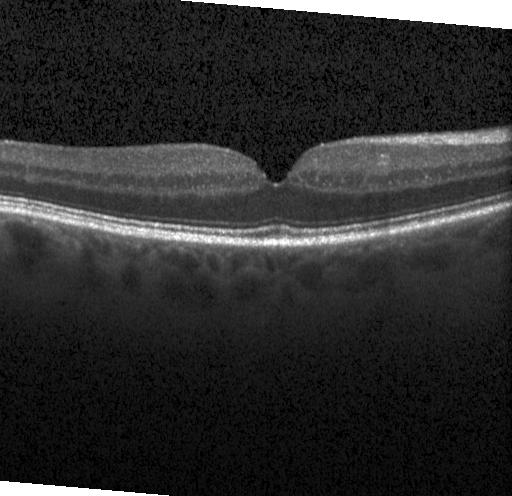
Through the macula; optical coherence tomography B-scan. Impression: no evidence of choroidal neovascularization, diabetic macular edema, or drusen.